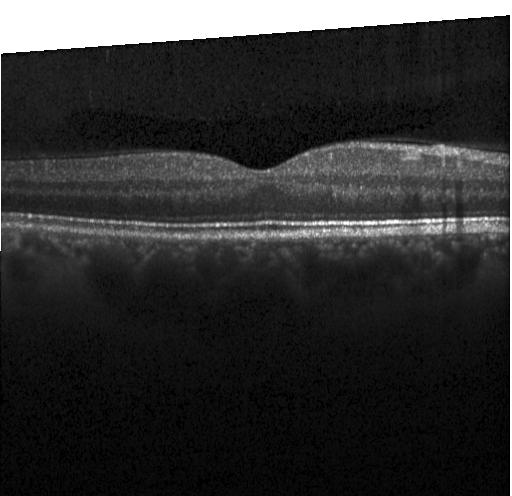

Acquired on a Heidelberg Spectralis. Retinal OCT B-scan. Through the macula. SD-OCT
Dx: no evidence of choroidal neovascularization, diabetic macular edema, or drusen.